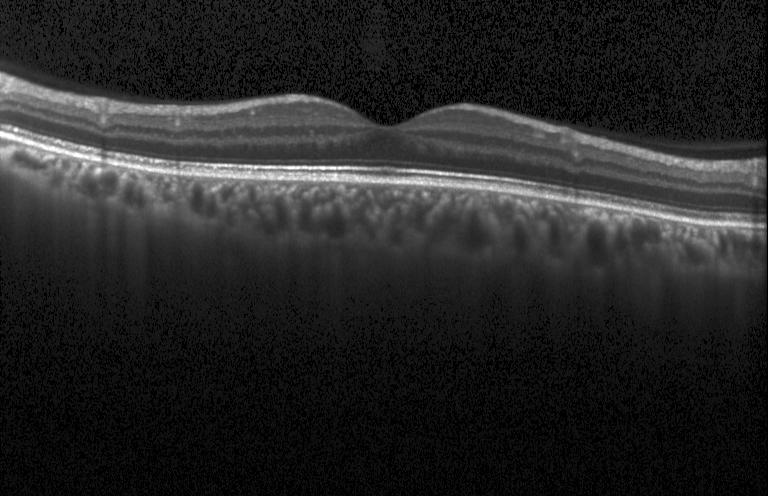

SD-OCT. Through the macula. OCT B-scan
Macular OCT: neither CNV, DME, nor drusen.